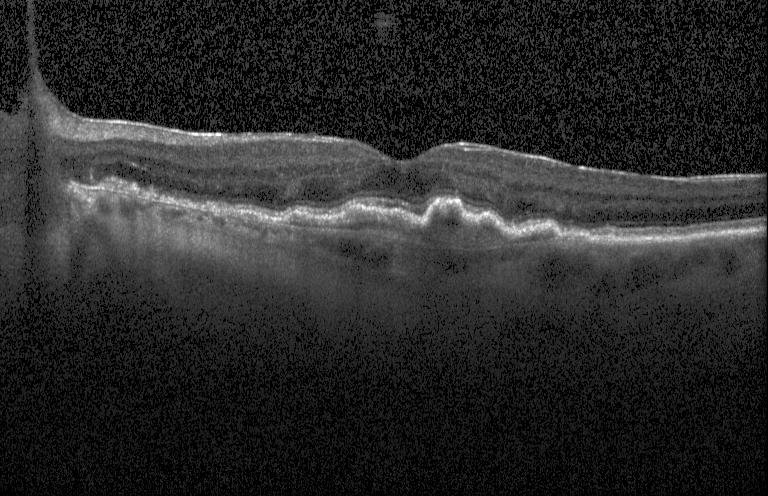 Dx: choroidal neovascularization (CNV).